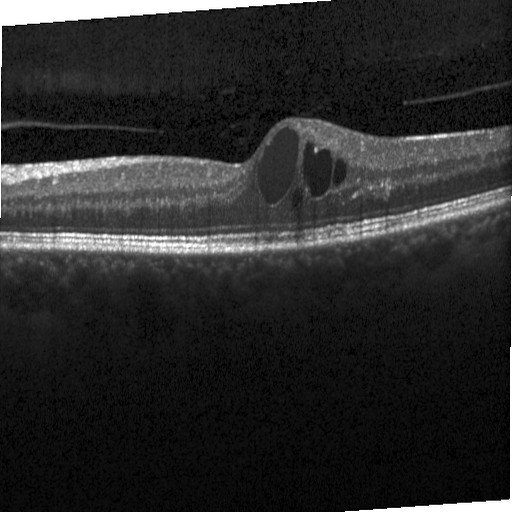 OCT line scan.
Impression: DME.